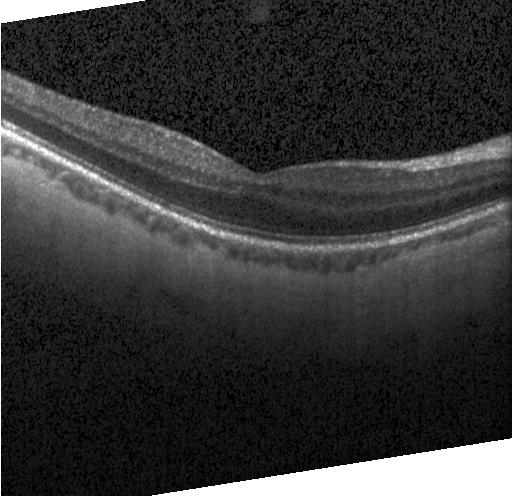

The scan shows no evidence of choroidal neovascularization, diabetic macular edema, or drusen.